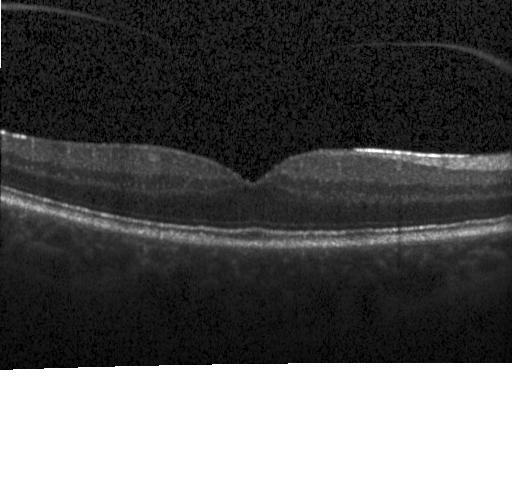 OCT finding: no evidence of choroidal neovascularization, diabetic macular edema, or drusen.